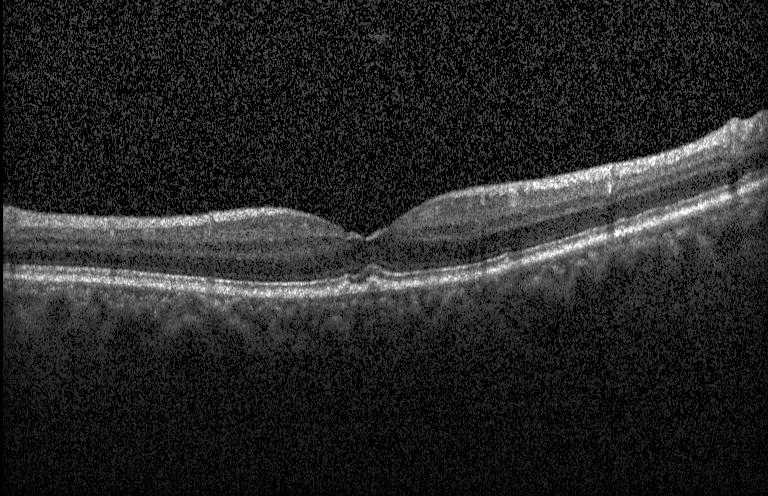

Macular OCT demonstrating sub-RPE drusenoid deposits.